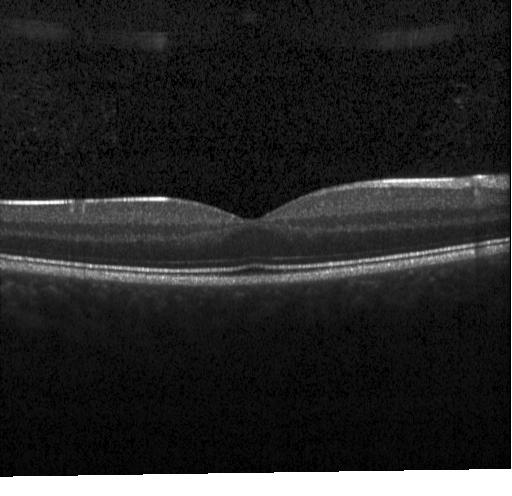 Retinal OCT cross-section
Dx: no CNV, DME, or drusen.